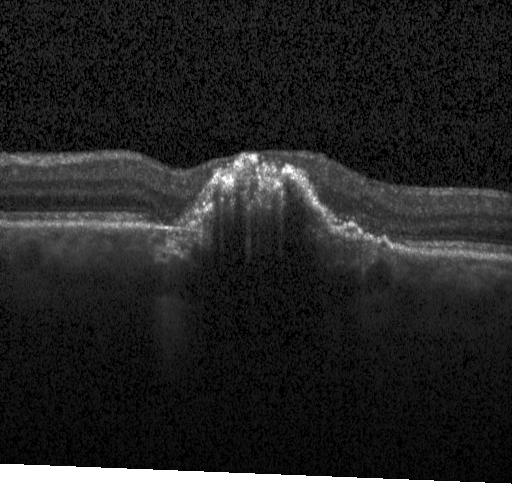

Optical coherence tomography B-scan.
Impression: a choroidal neovascular membrane.